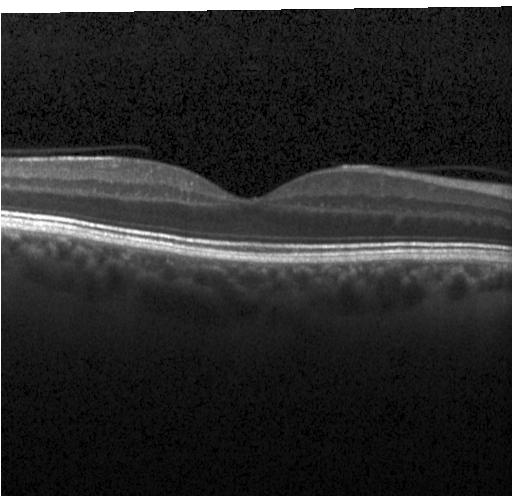

Diagnosis: no evidence of choroidal neovascularization, diabetic macular edema, or drusen.